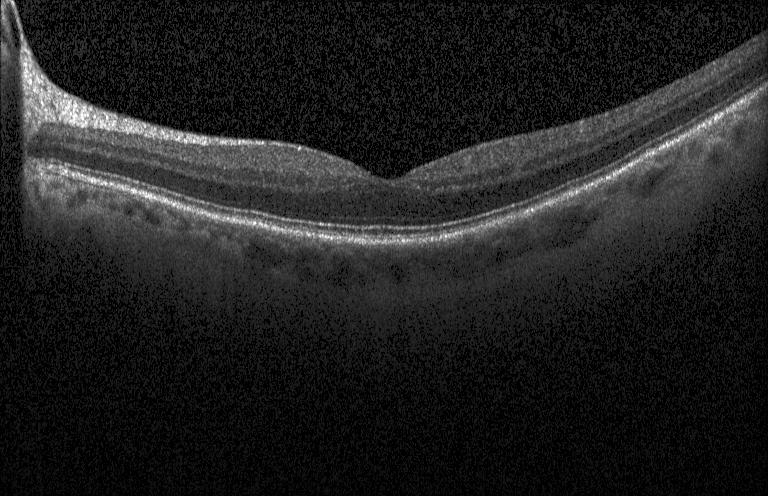 Diagnosis: no CNV, no DME, and no drusen.